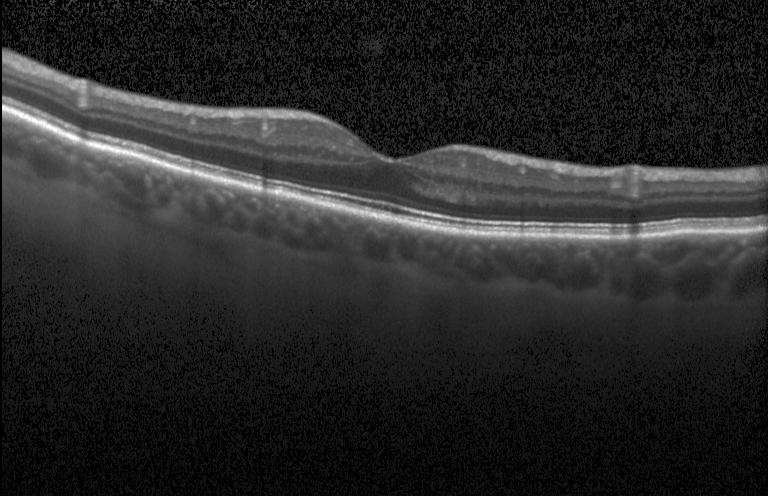 Optical coherence tomography B-scan
Finding: no evidence of CNV, DME, or drusen.